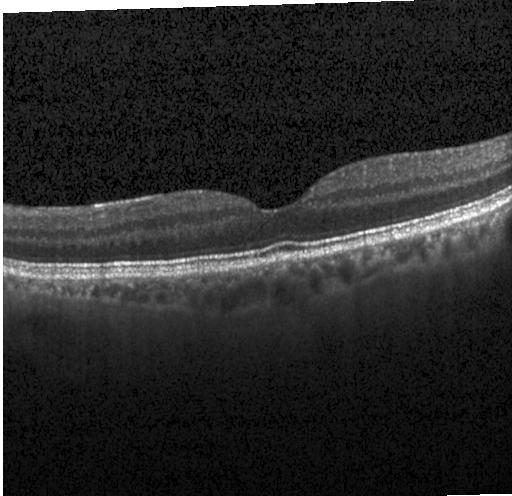

Impression: neither CNV, DME, nor drusen.